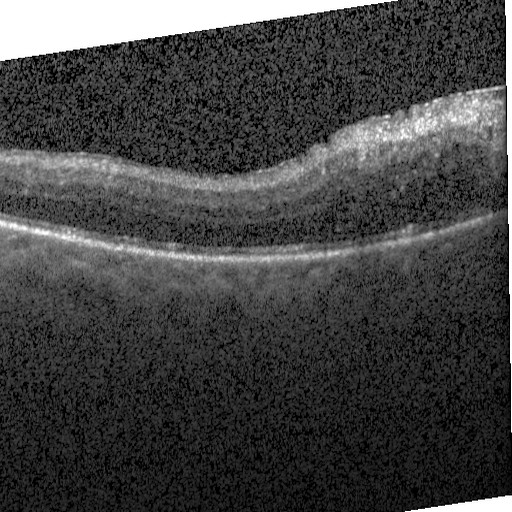

Retinal OCT cross-section.
Impression: diabetic macular edema (DME).